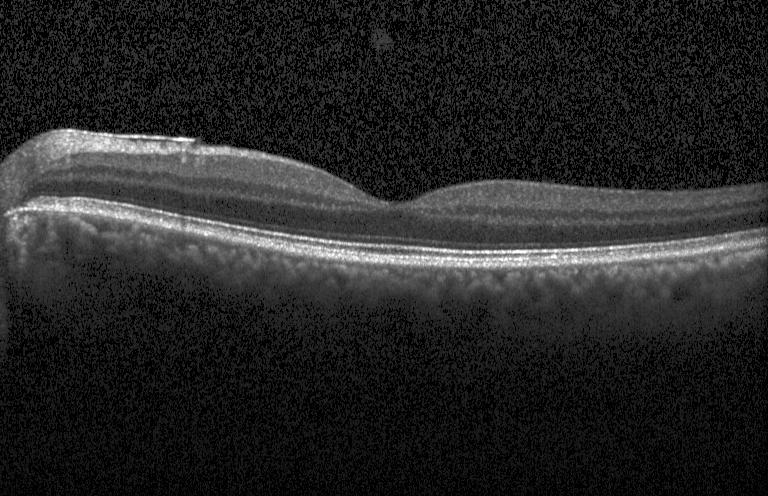

Retinal OCT B-scan; spectral-domain optical coherence tomography
Finding: neither choroidal neovascularization, diabetic macular edema, nor drusen.